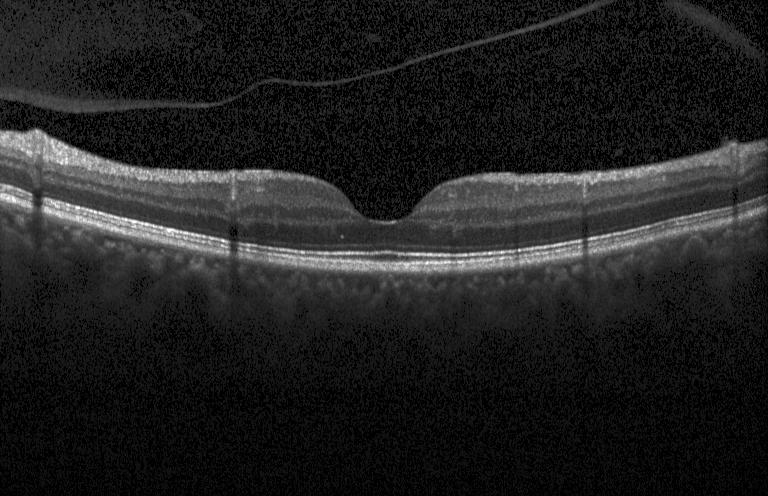 Optical coherence tomography B-scan · SD-OCT · Heidelberg Spectralis.
Finding: no CNV, DME, or drusen.